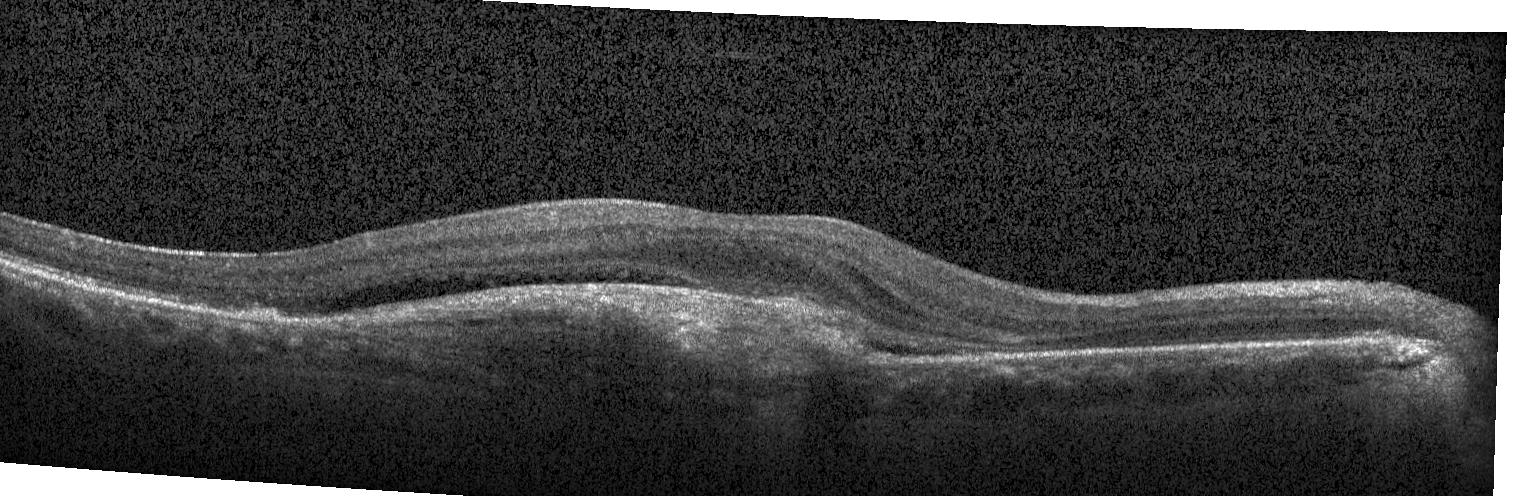

CNV.